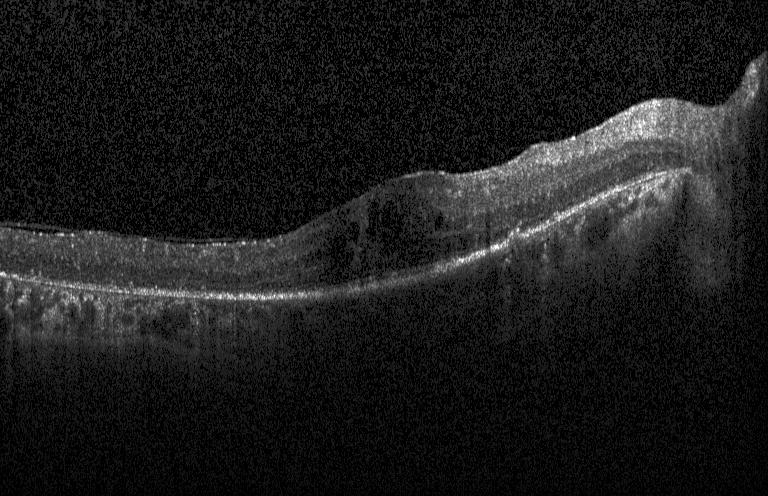 The scan shows DME.